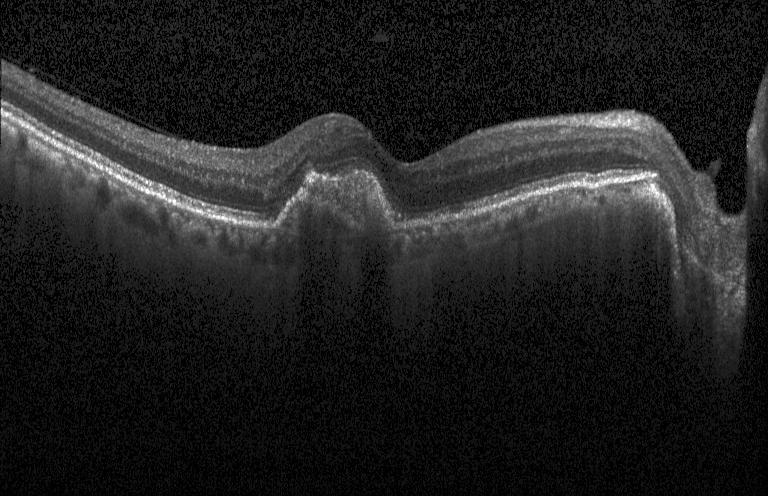

The scan shows choroidal neovascularization (CNV).